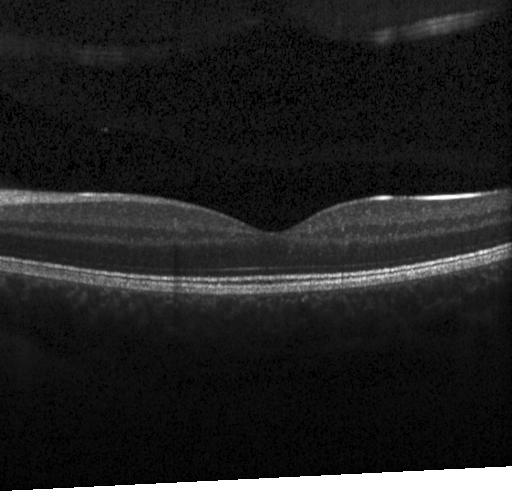

Macular OCT demonstrating no evidence of CNV, DME, or drusen.